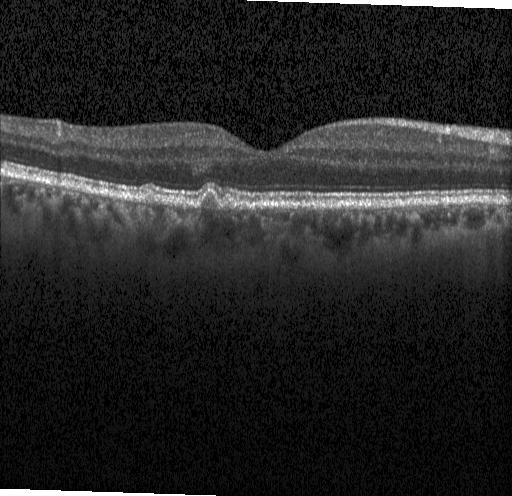 Spectral-domain OCT; instrument: Heidelberg Spectralis; optical coherence tomography B-scan; horizontal scan through the fovea
This B-scan demonstrates sub-RPE drusenoid deposits.